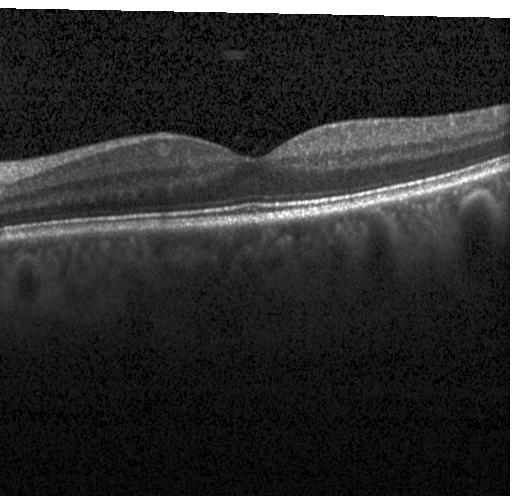
Spectral-domain OCT, horizontal scan through the fovea, acquired on a Heidelberg Spectralis, OCT B-scan. Impression: no evidence of CNV, DME, or drusen.